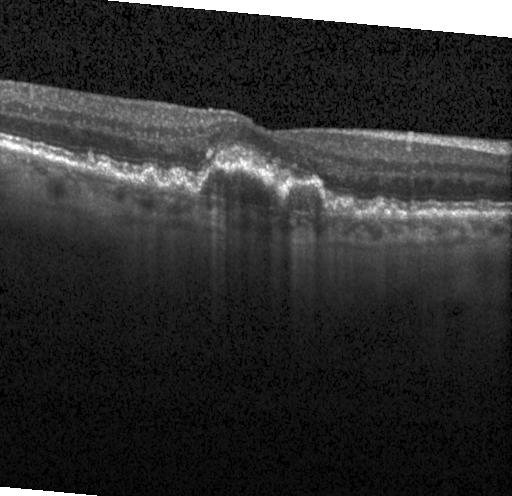

Diagnosis: a choroidal neovascular membrane.